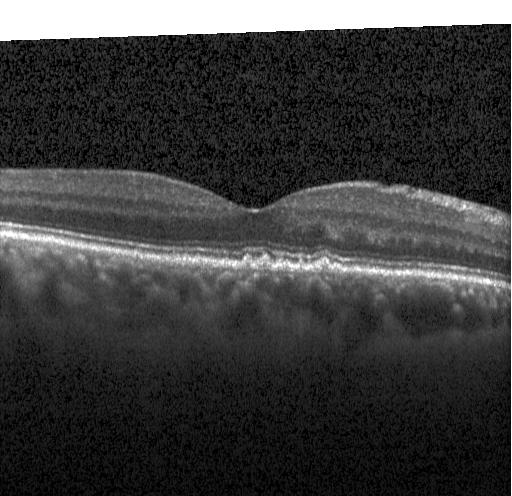
Diagnosis: multiple drusen.